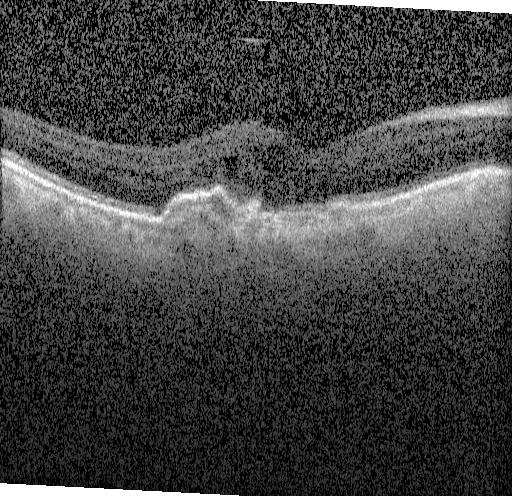 OCT B-scan.
Impression: a choroidal neovascular membrane.